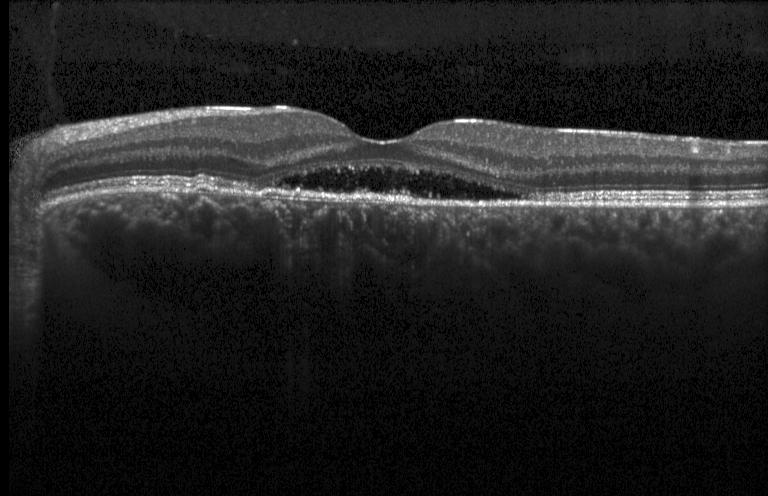

Retinal OCT B-scan. Heidelberg Spectralis. Spectral-domain OCT
Impression: CNV.